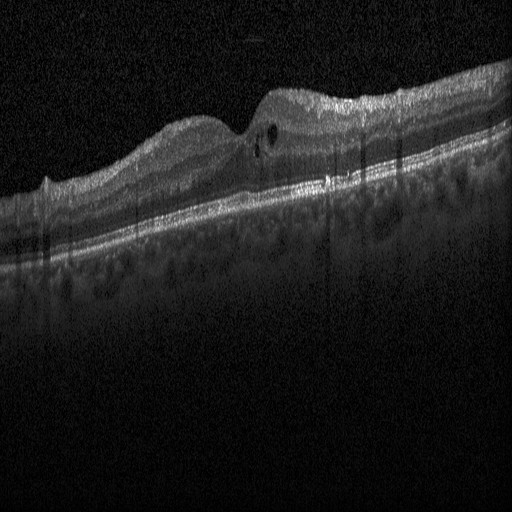
Optical coherence tomography B-scan · instrument: Heidelberg Spectralis.
Diabetic macular edema (DME).